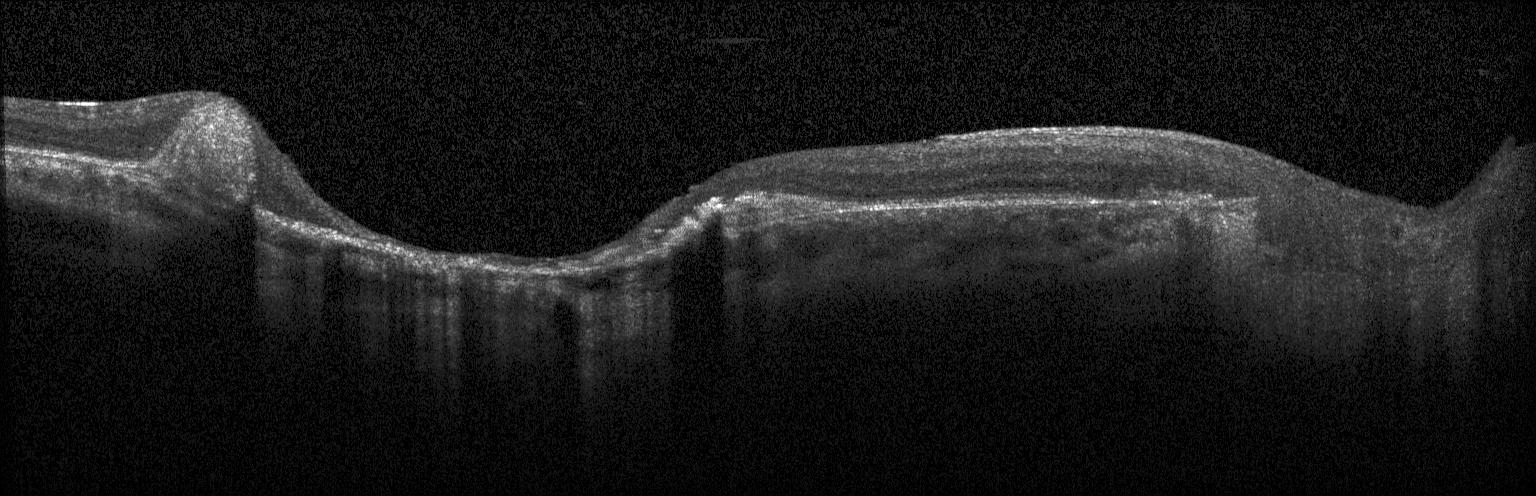 Finding: a choroidal neovascular membrane.